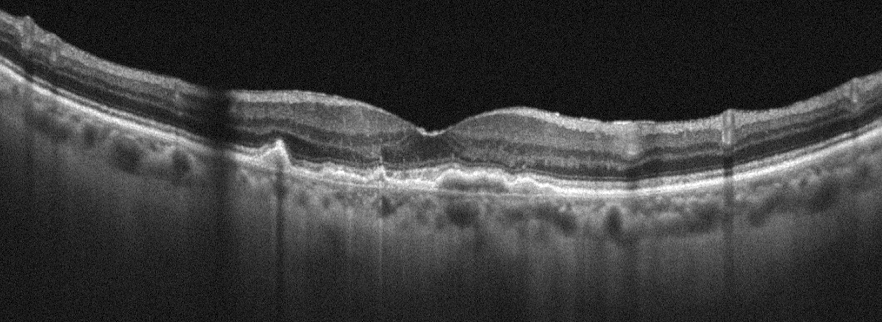

Right eye · optical coherence tomography scan — Age-related macular degeneration (AMD).